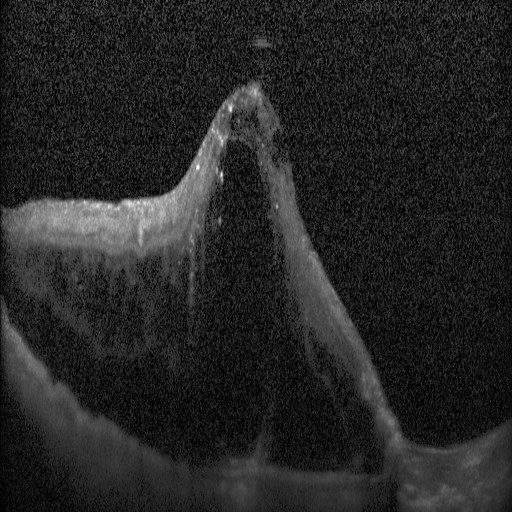
Spectral-domain optical coherence tomography · optical coherence tomography scan — Diagnosis: DME.